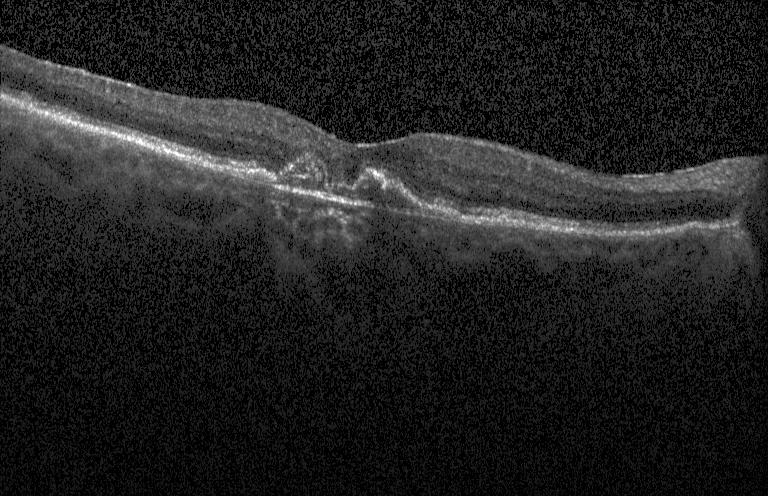
Optical coherence tomography B-scan. Through the macula — The scan shows choroidal neovascularization (CNV).